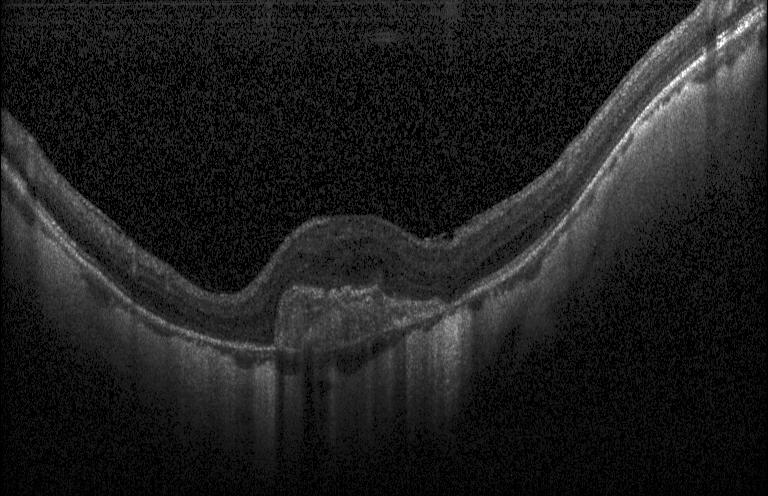 OCT B-scan showing choroidal neovascularization.